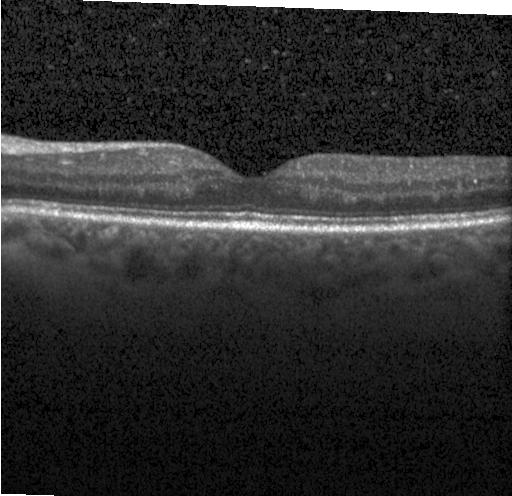

OCT line scan
Finding: no choroidal neovascularization, no diabetic macular edema, and no drusen.